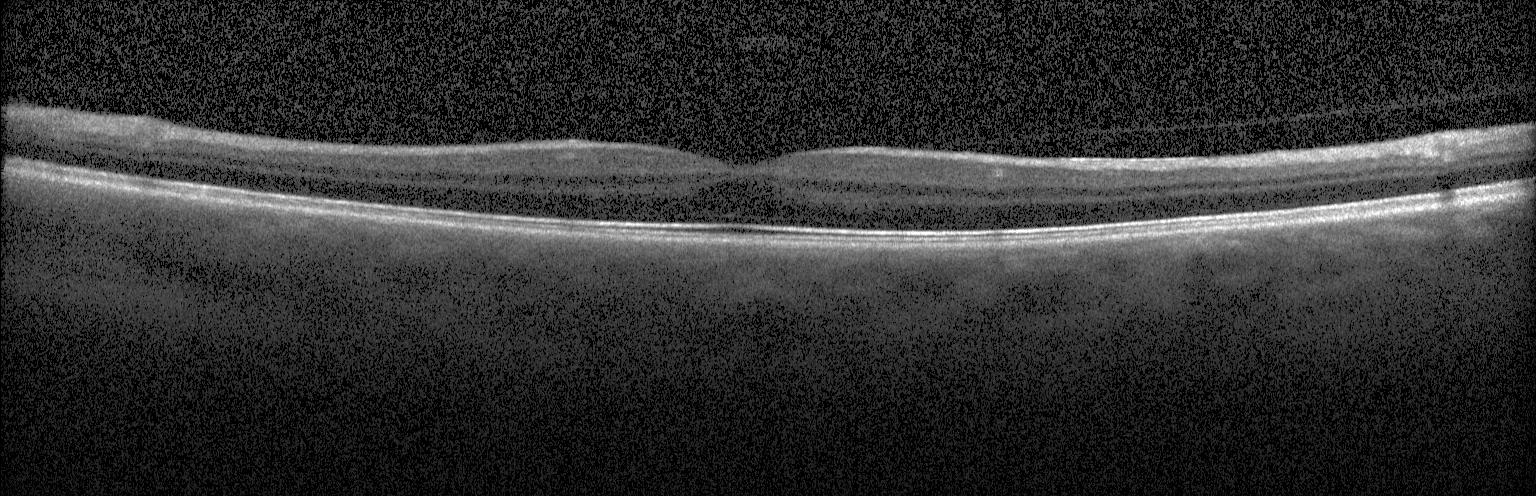

Diagnosis: no choroidal neovascularization, no diabetic macular edema, and no drusen.